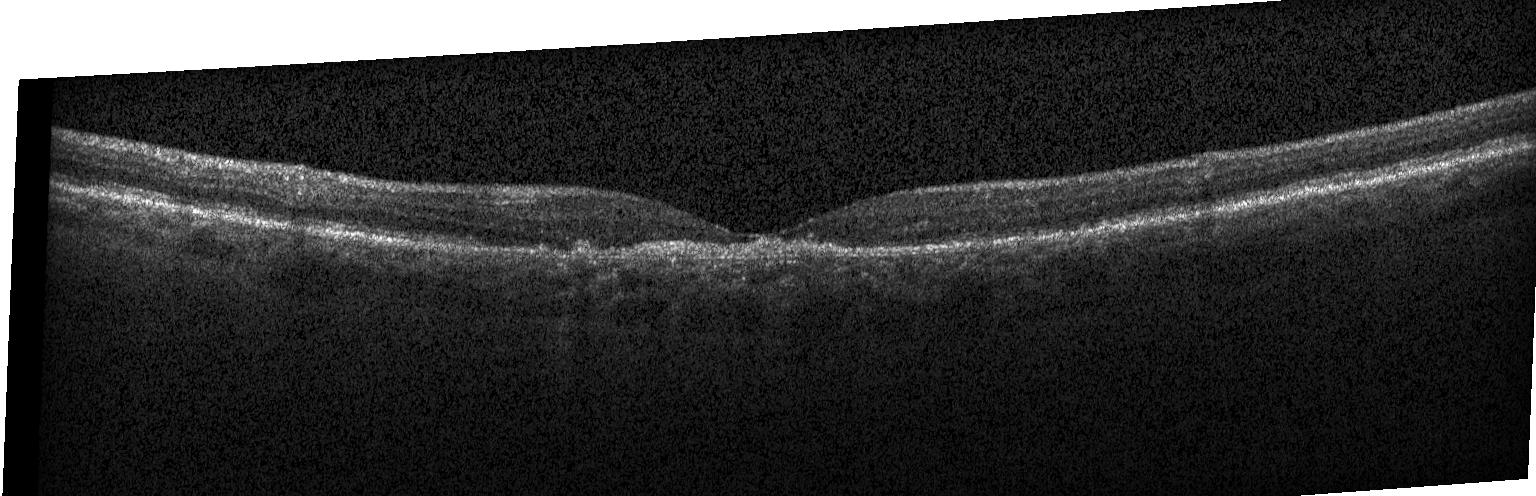
Retinal OCT B-scan. Dx: CNV.